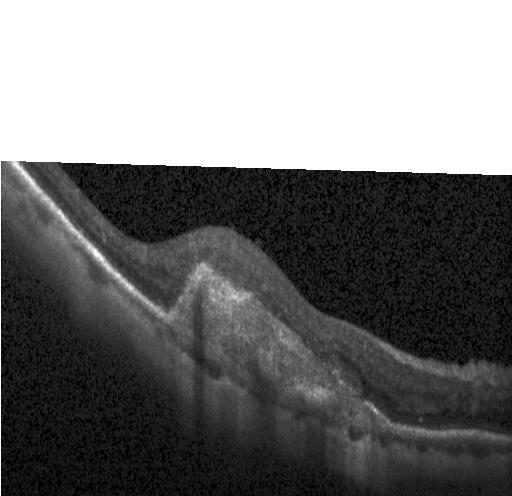
Through the macula, spectral-domain optical coherence tomography, Heidelberg Spectralis OCT system, retinal OCT cross-section. Dx: choroidal neovascularization.